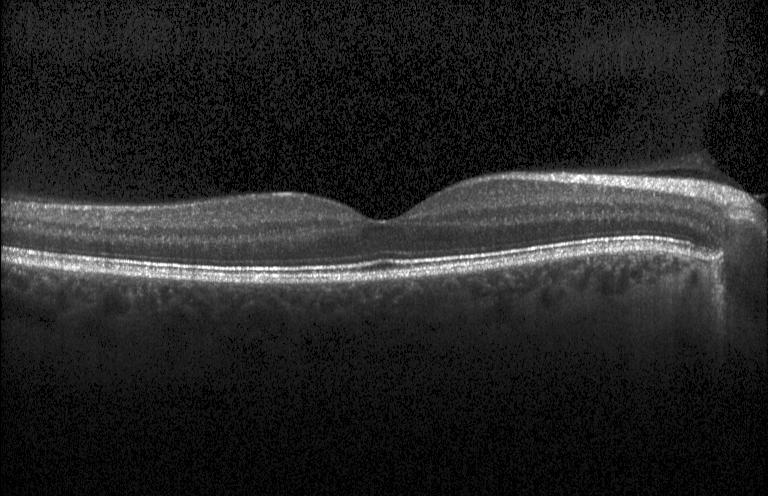 Macular OCT: no choroidal neovascularization, no diabetic macular edema, and no drusen.